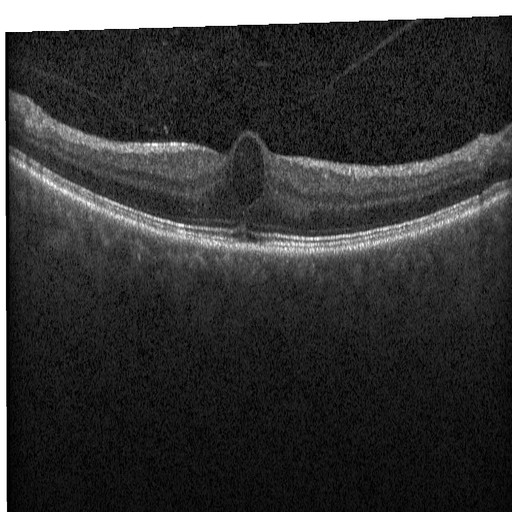

Macular OCT: DME.